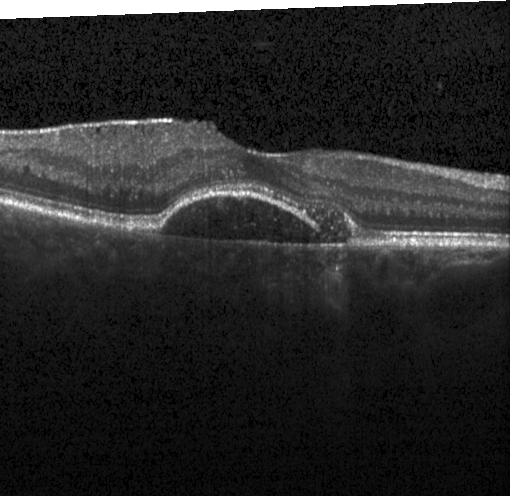 Diagnosis: choroidal neovascularization.